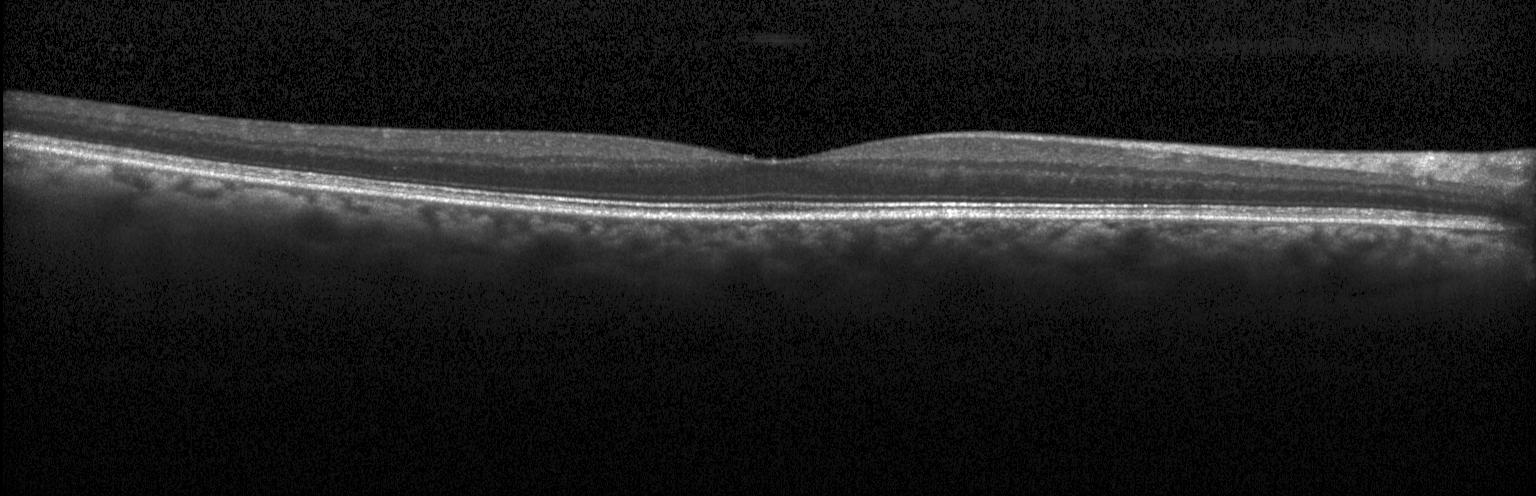

This B-scan demonstrates no choroidal neovascularization, diabetic macular edema, or drusen.